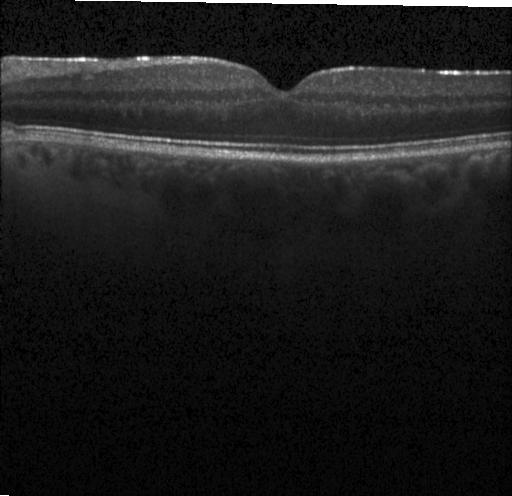

Heidelberg Spectralis OCT system · OCT line scan · macular scan — Finding: no choroidal neovascularization, diabetic macular edema, or drusen.